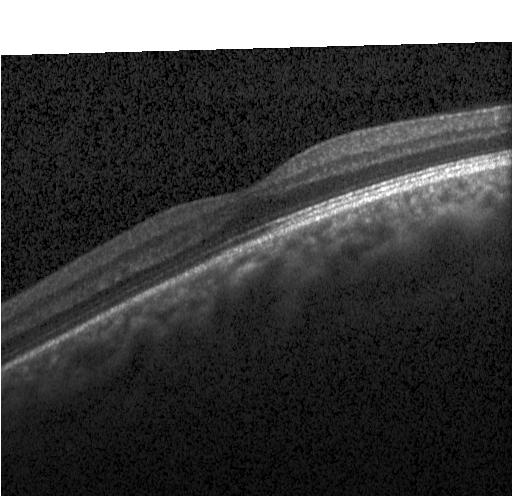 OCT B-scan
No choroidal neovascularization, no diabetic macular edema, and no drusen.